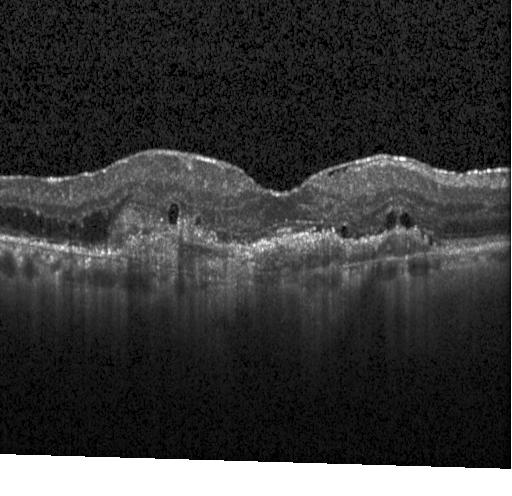 SD-OCT, retinal OCT B-scan.
Impression: CNV.